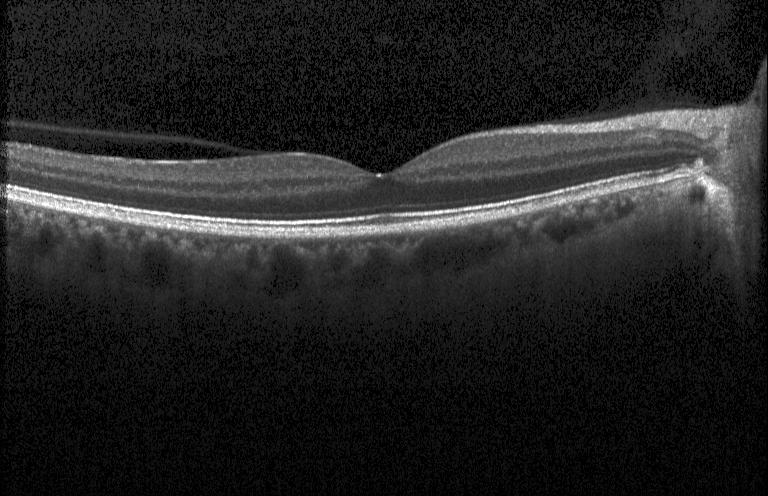
Retinal OCT B-scan · Heidelberg Spectralis. No choroidal neovascularization, diabetic macular edema, or drusen.